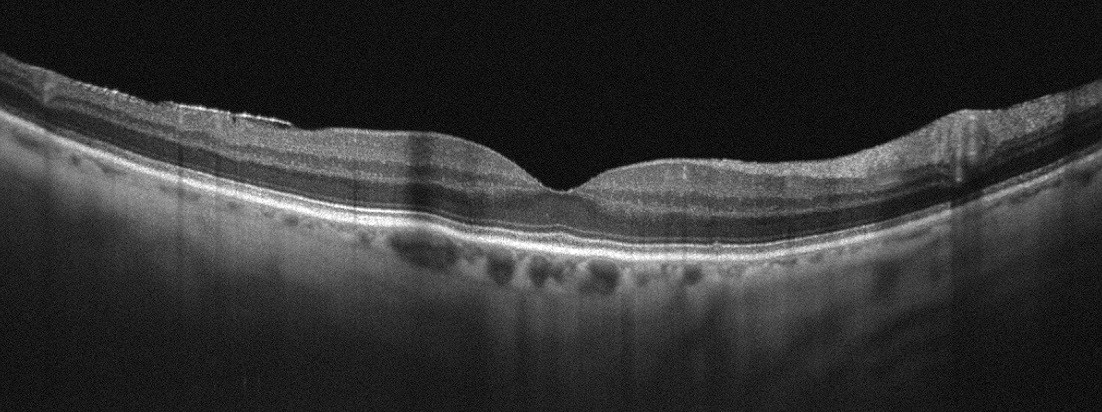
Retinal OCT cross-section
Impression: epiretinal membrane (ERM).